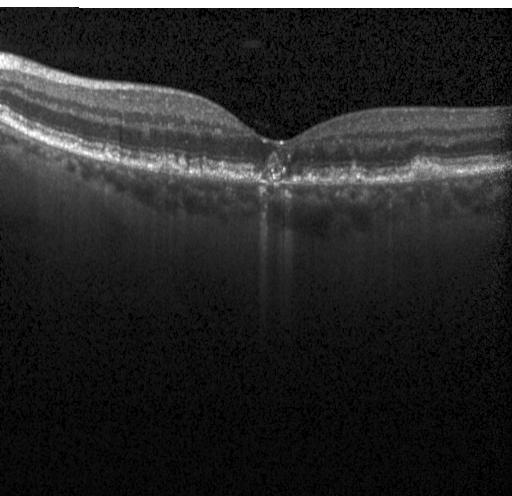

This B-scan demonstrates CNV.